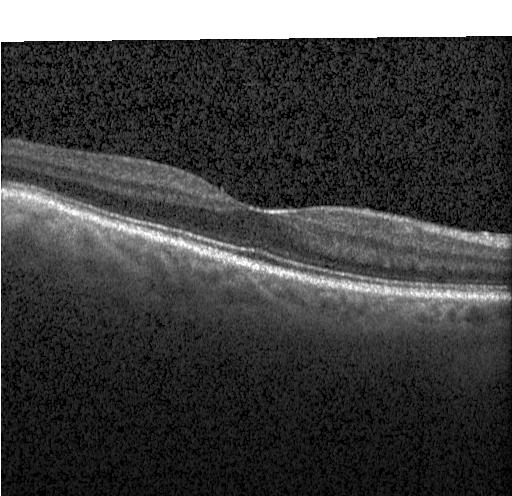

Horizontal scan through the fovea · optical coherence tomography scan.
Assessment: neither choroidal neovascularization, diabetic macular edema, nor drusen.